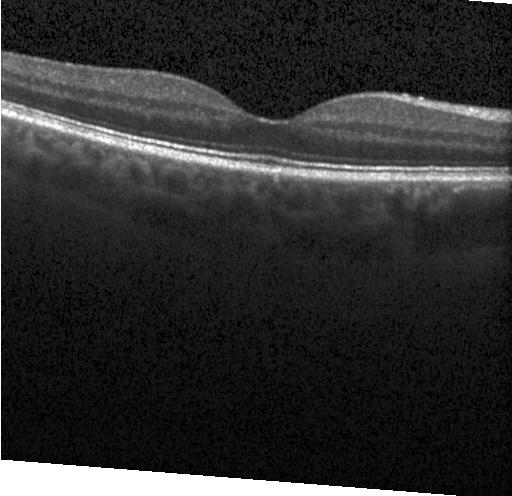

Optical coherence tomography B-scan. Instrument: Heidelberg Spectralis
Finding: neither CNV, DME, nor drusen.